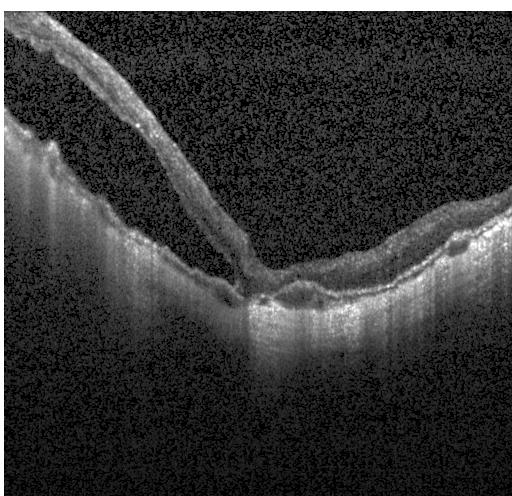

Diagnosis: choroidal neovascularization.